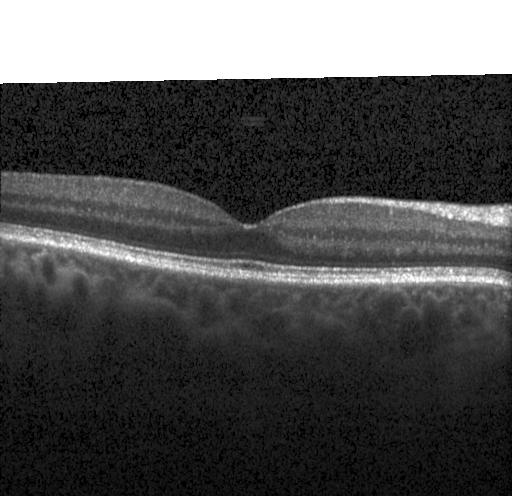

Heidelberg Spectralis OCT system, optical coherence tomography B-scan, centered on the fovea, SD-OCT — Assessment: no choroidal neovascularization, no diabetic macular edema, and no drusen.